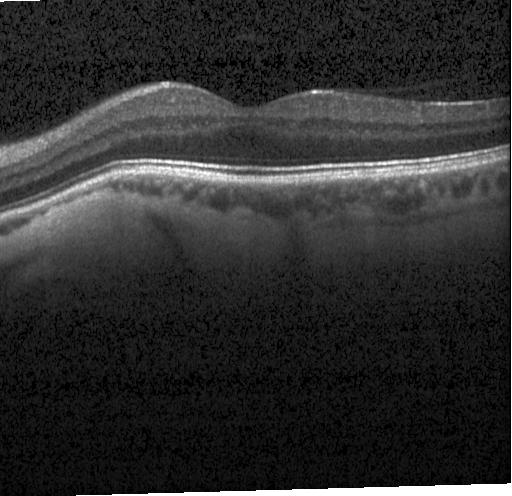
Optical coherence tomography scan, spectral-domain optical coherence tomography — OCT finding: no CNV, DME, or drusen.